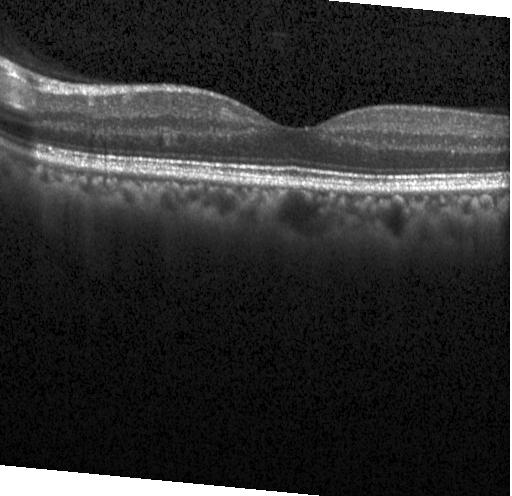

OCT B-scan. SD-OCT
Diagnosis: no choroidal neovascularization, no diabetic macular edema, and no drusen.